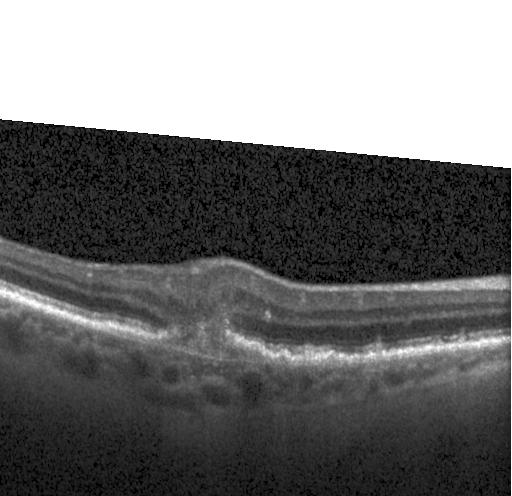
OCT B-scan. Heidelberg Spectralis. Fovea-centered. Spectral-domain optical coherence tomography. Macular OCT: a choroidal neovascular membrane.